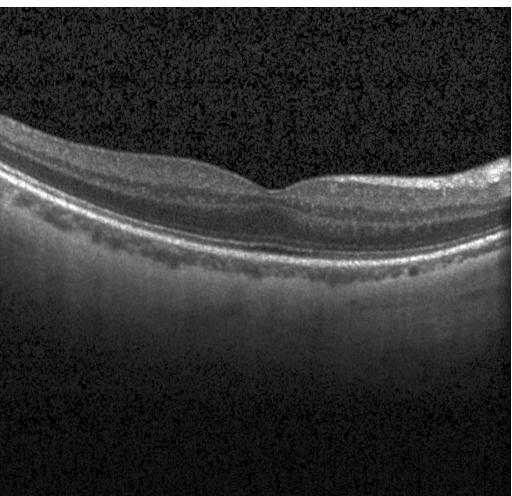

Spectral-domain OCT; centered on the fovea; optical coherence tomography B-scan — This B-scan demonstrates no choroidal neovascularization, diabetic macular edema, or drusen.